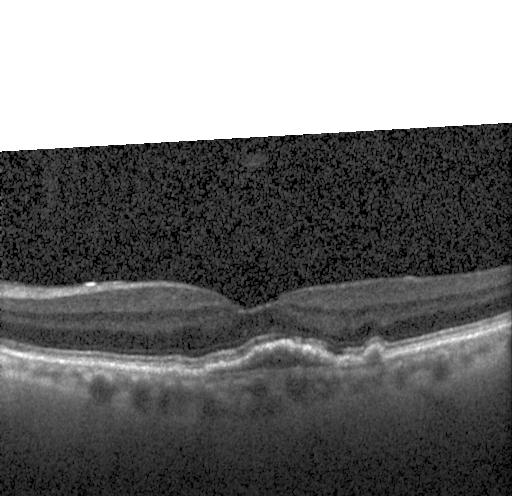
Impression: a choroidal neovascular membrane.